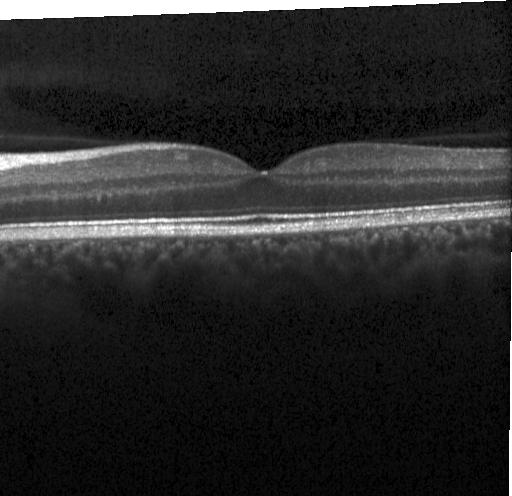
OCT B-scan.
Finding: no evidence of choroidal neovascularization, diabetic macular edema, or drusen.